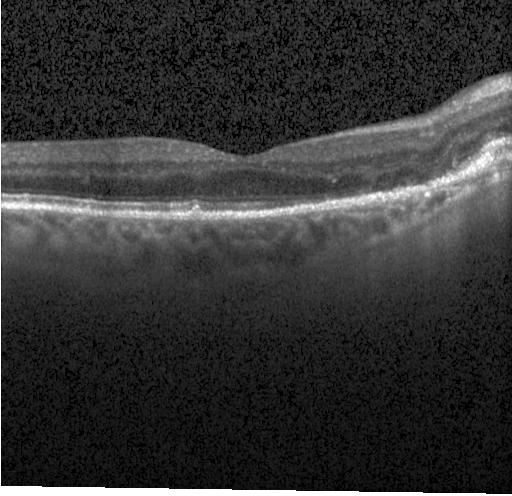
Acquired on a Heidelberg Spectralis · macular scan · OCT B-scan · spectral-domain OCT — Diagnosis: a choroidal neovascular membrane.